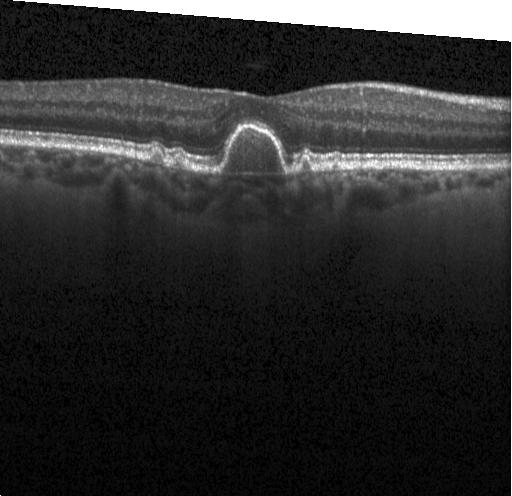
Spectral-domain optical coherence tomography, OCT line scan. The scan shows a choroidal neovascular membrane.